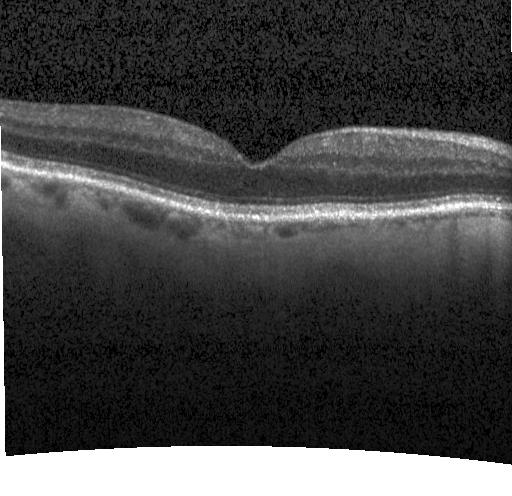
Optical coherence tomography B-scan; spectral-domain optical coherence tomography; through the macula — Assessment: neither choroidal neovascularization, diabetic macular edema, nor drusen.